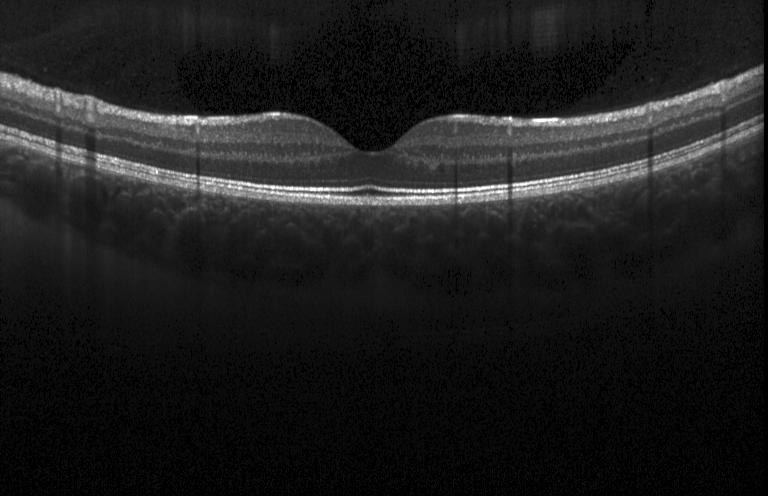
Finding: neither choroidal neovascularization, diabetic macular edema, nor drusen.